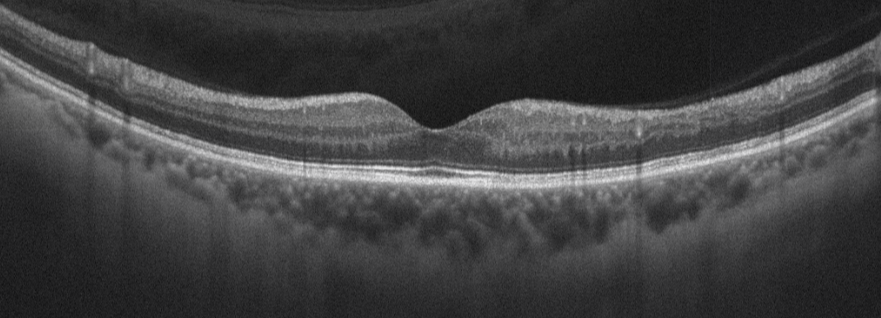
Optovue Avanti RTVue XR; optical coherence tomography scan; fovea-centered. The scan shows no evidence of AMD, DME, ERM, RAO, RVO, or VID.